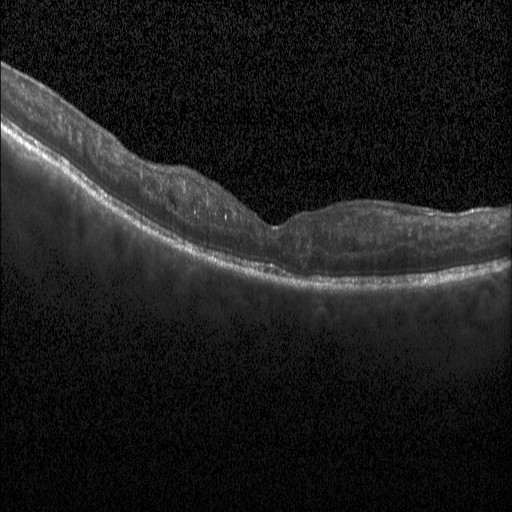
Spectral-domain OCT · retinal OCT B-scan · acquired on a Heidelberg Spectralis · macular scan
Impression: diabetic macular edema.